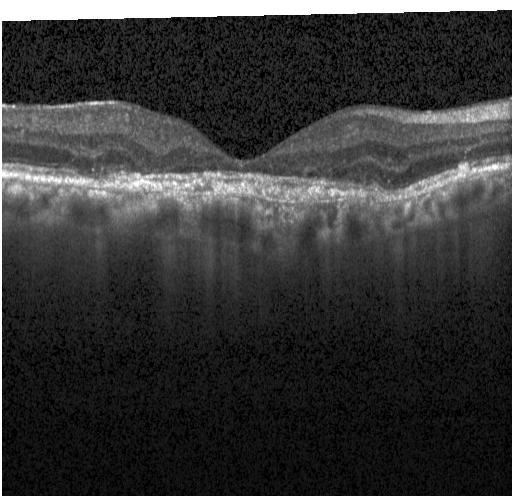 OCT B-scan. Macular OCT: CNV.